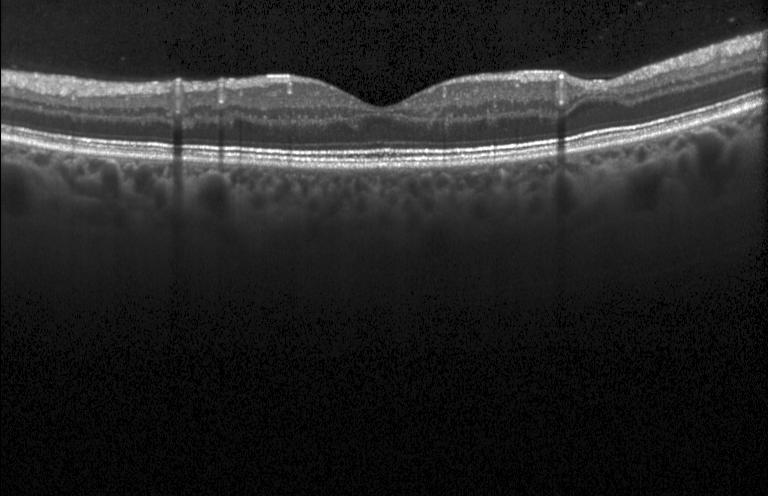 Finding: neither CNV, DME, nor drusen.